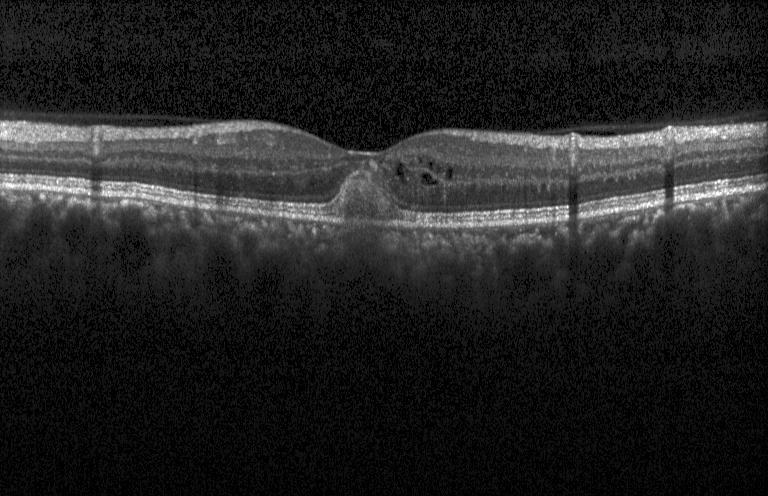 OCT B-scan showing a choroidal neovascular membrane.